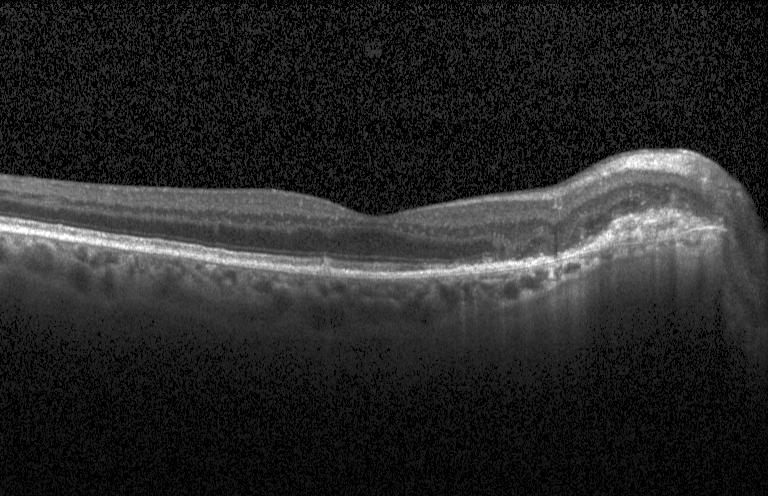 Centered on the fovea; OCT line scan.
Diagnosis: a choroidal neovascular membrane.